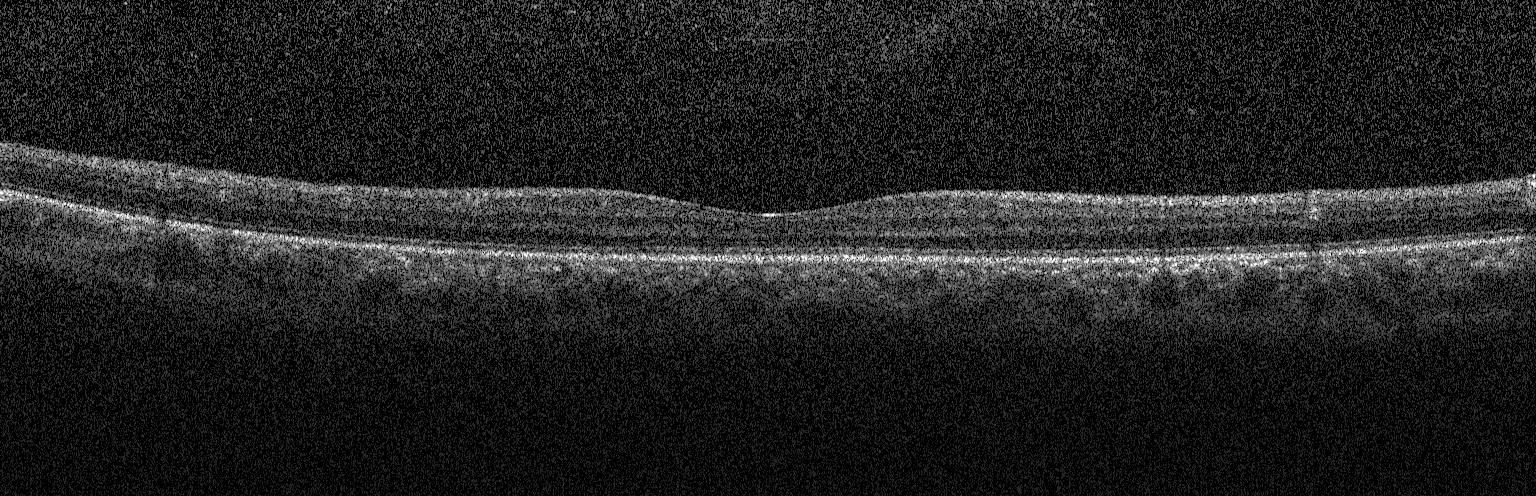
Macular scan · instrument: Heidelberg Spectralis · spectral-domain OCT · optical coherence tomography B-scan — Dx: no evidence of choroidal neovascularization, diabetic macular edema, or drusen.